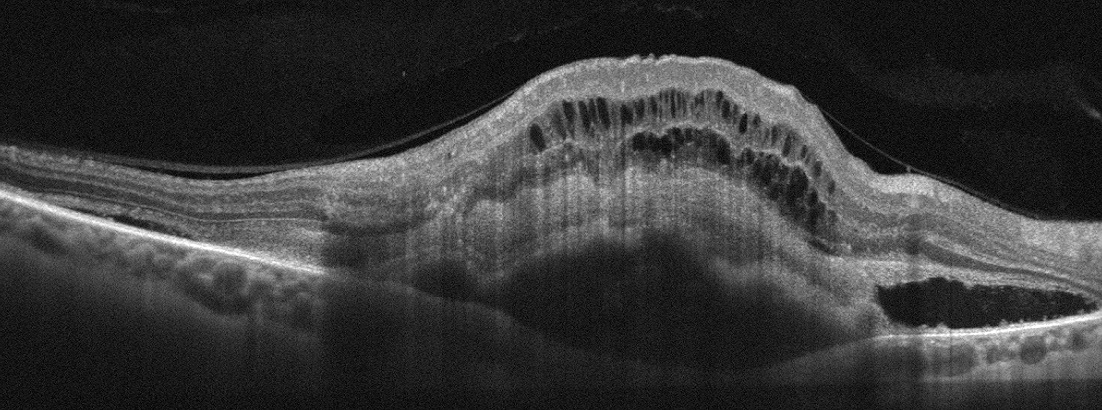 Spectral-domain OCT B-scan: age-related macular degeneration.